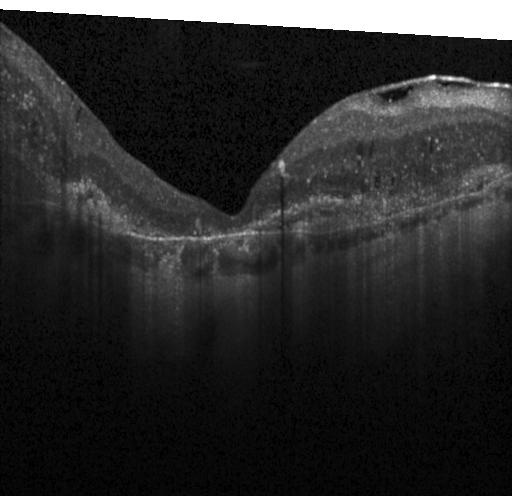 OCT line scan. The scan shows choroidal neovascularization (CNV).